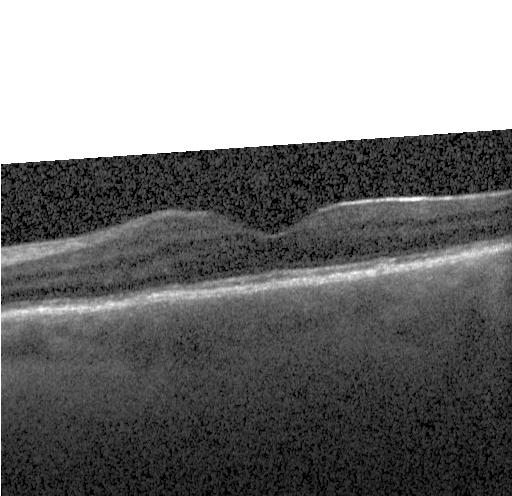

Retinal OCT cross-section; horizontal scan through the fovea; SD-OCT; Heidelberg Spectralis — OCT finding: no CNV, DME, or drusen.